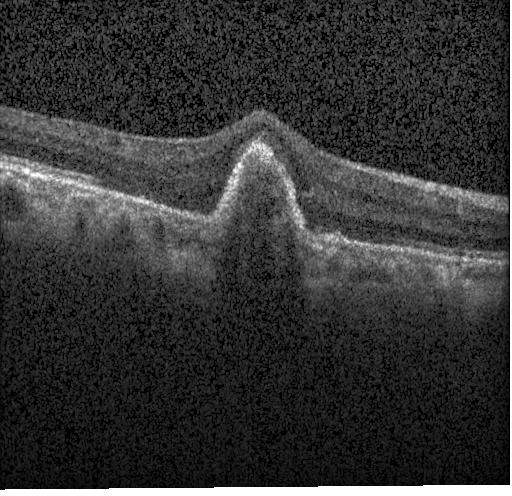

Retinal OCT B-scan · macular scan.
Diagnosis: choroidal neovascularization.